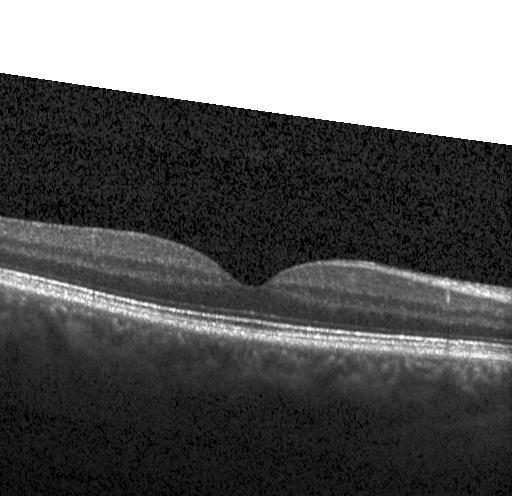 Retinal OCT B-scan. Finding: no choroidal neovascularization, diabetic macular edema, or drusen.